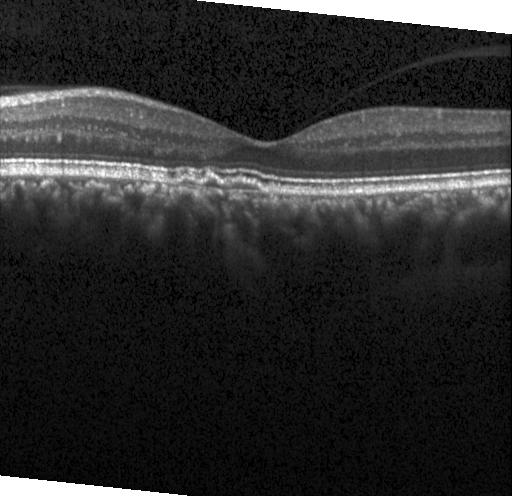

Retinal OCT B-scan, centered on the fovea — Diagnosis: sub-RPE drusenoid deposits.